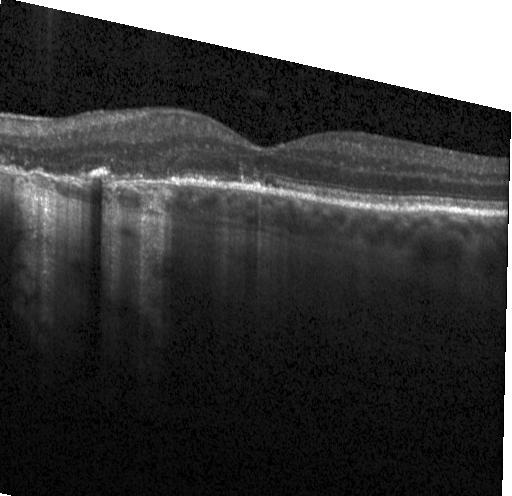 Macular OCT: CNV.